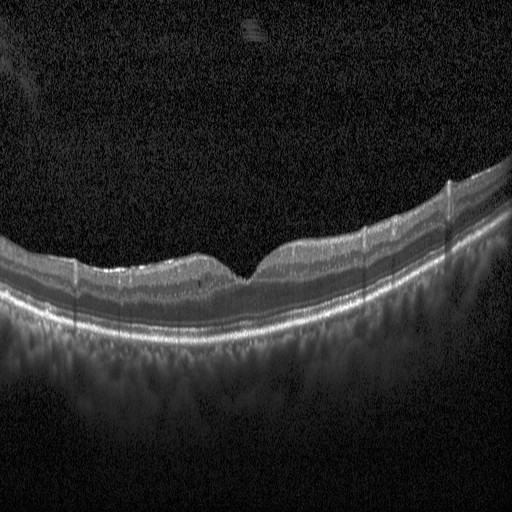 Acquired on a Heidelberg Spectralis, spectral-domain optical coherence tomography, through the macula, optical coherence tomography scan.
This B-scan demonstrates diabetic macular edema (DME).